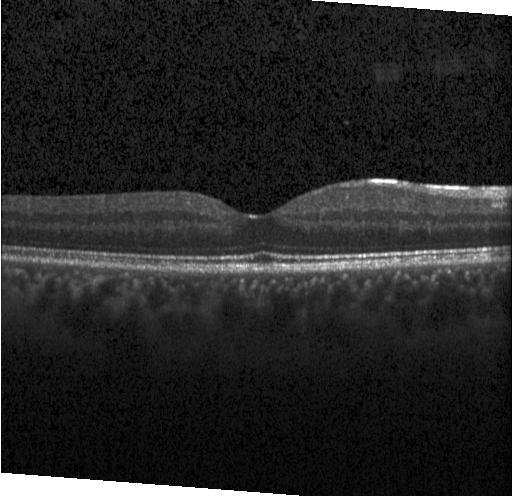
Optical coherence tomography B-scan · spectral-domain OCT · acquired on a Heidelberg Spectralis · centered on the fovea.
Finding: no CNV, no DME, and no drusen.